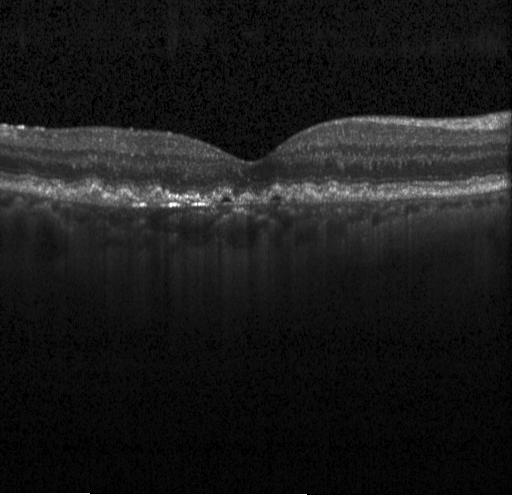
Instrument: Heidelberg Spectralis. SD-OCT. Retinal OCT cross-section.
Finding: a choroidal neovascular membrane.